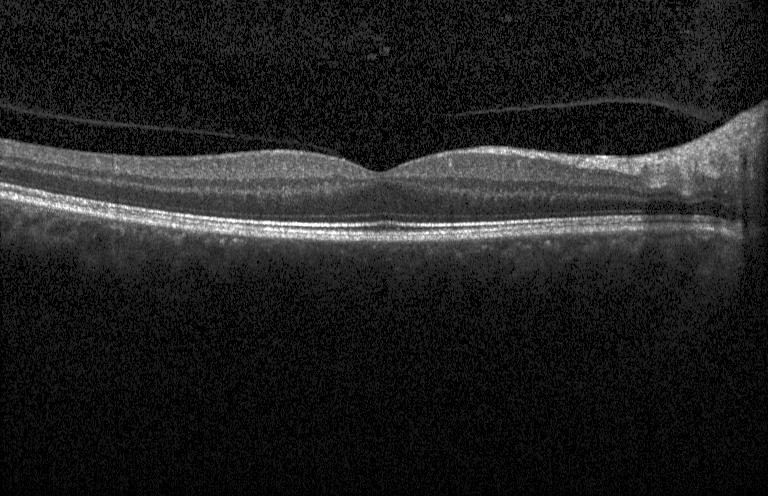

Instrument: Heidelberg Spectralis, OCT B-scan, spectral-domain optical coherence tomography.
Diagnosis: neither choroidal neovascularization, diabetic macular edema, nor drusen.